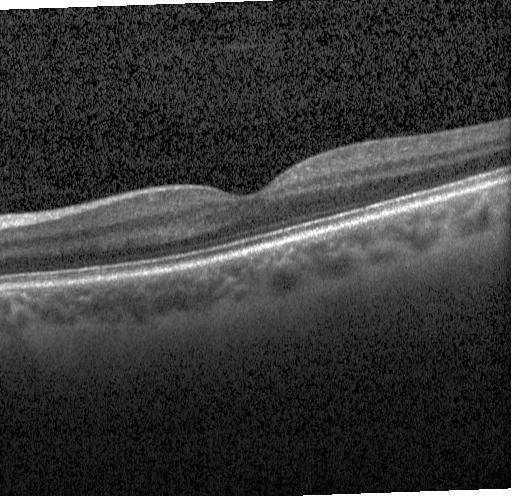
Retinal OCT cross-section · spectral-domain OCT. Macular OCT: no evidence of choroidal neovascularization, diabetic macular edema, or drusen.